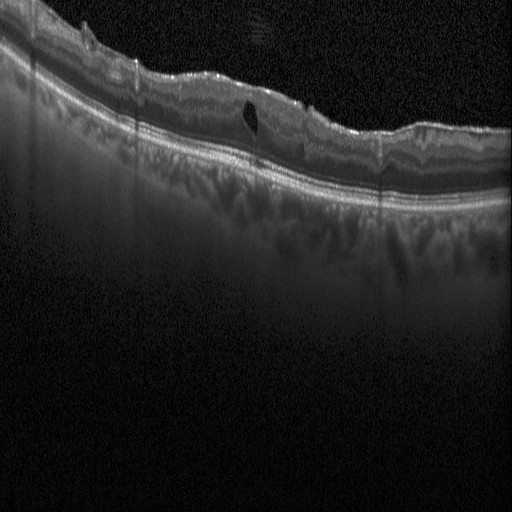 Spectral-domain optical coherence tomography, retinal OCT B-scan, through the macula, Heidelberg Spectralis OCT system
OCT finding: diabetic macular edema (DME).